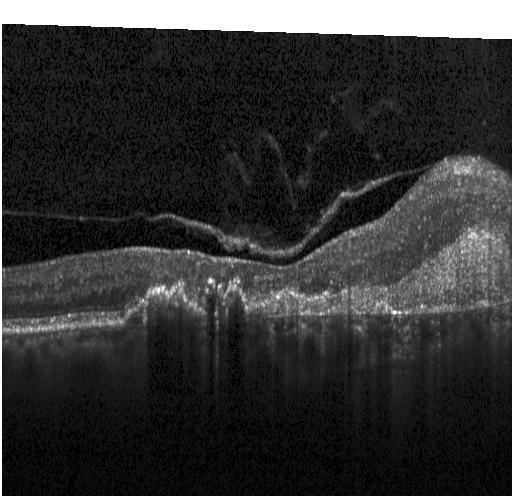 OCT line scan.
Impression: choroidal neovascularization (CNV).